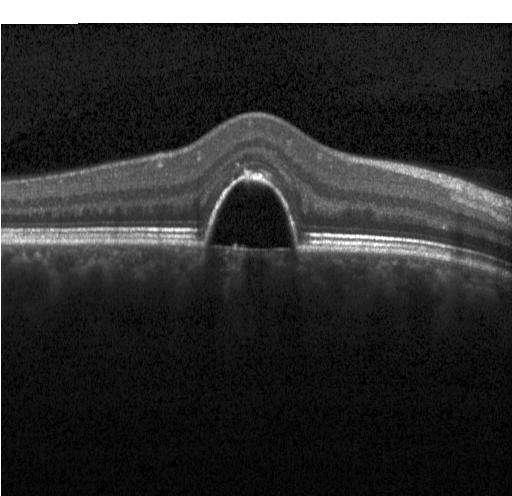
The scan shows a choroidal neovascular membrane.